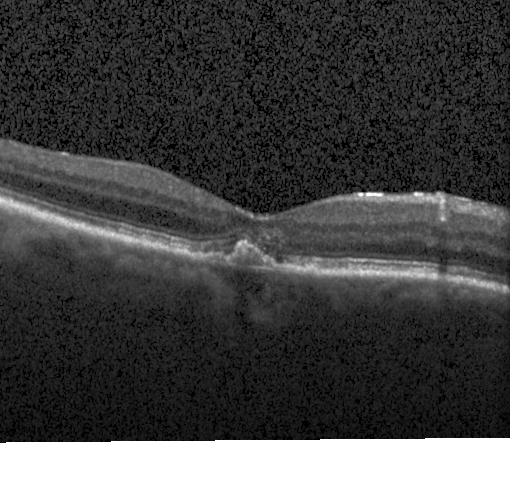 Through the macula. Retinal OCT cross-section. Heidelberg Spectralis OCT system. Spectral-domain optical coherence tomography.
Impression: choroidal neovascularization (CNV).